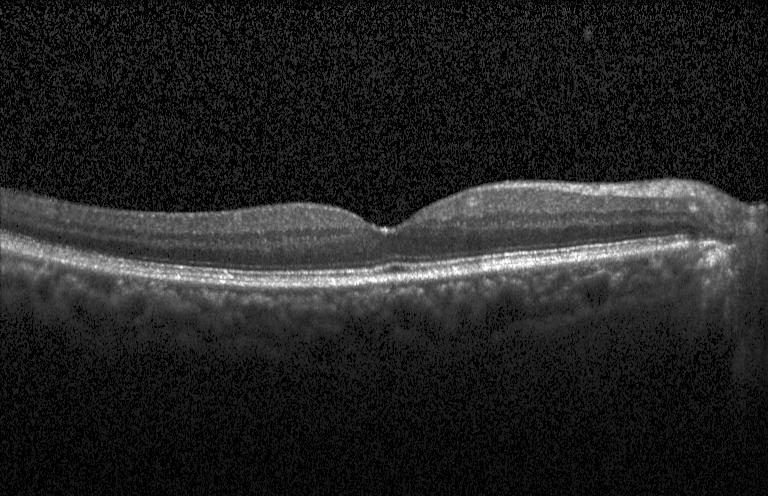

Retinal OCT cross-section showing neither choroidal neovascularization, diabetic macular edema, nor drusen.